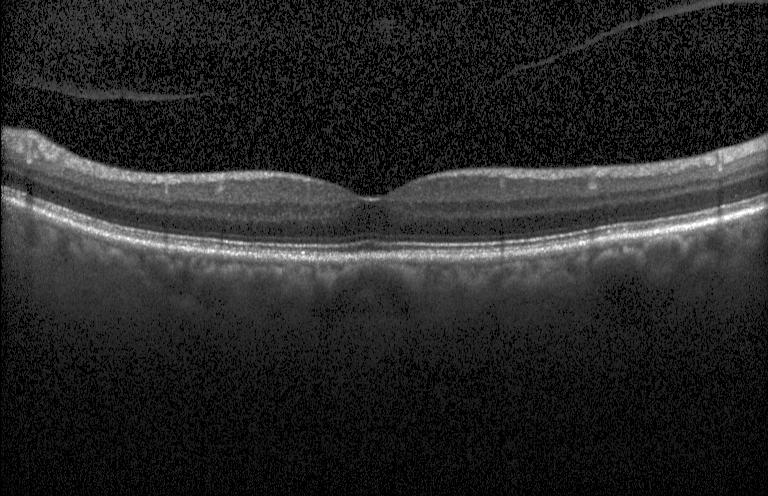

Diagnosis: no choroidal neovascularization, diabetic macular edema, or drusen.